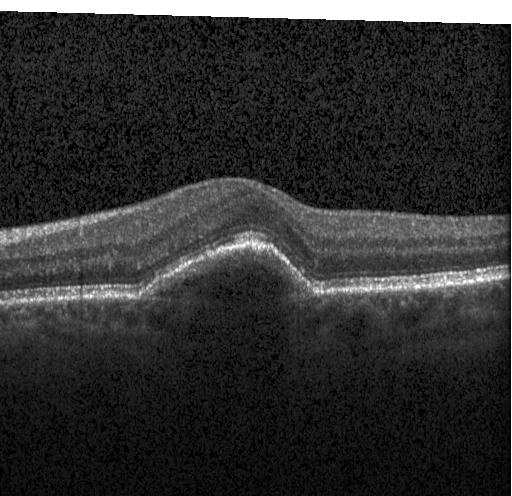
OCT finding: a choroidal neovascular membrane.